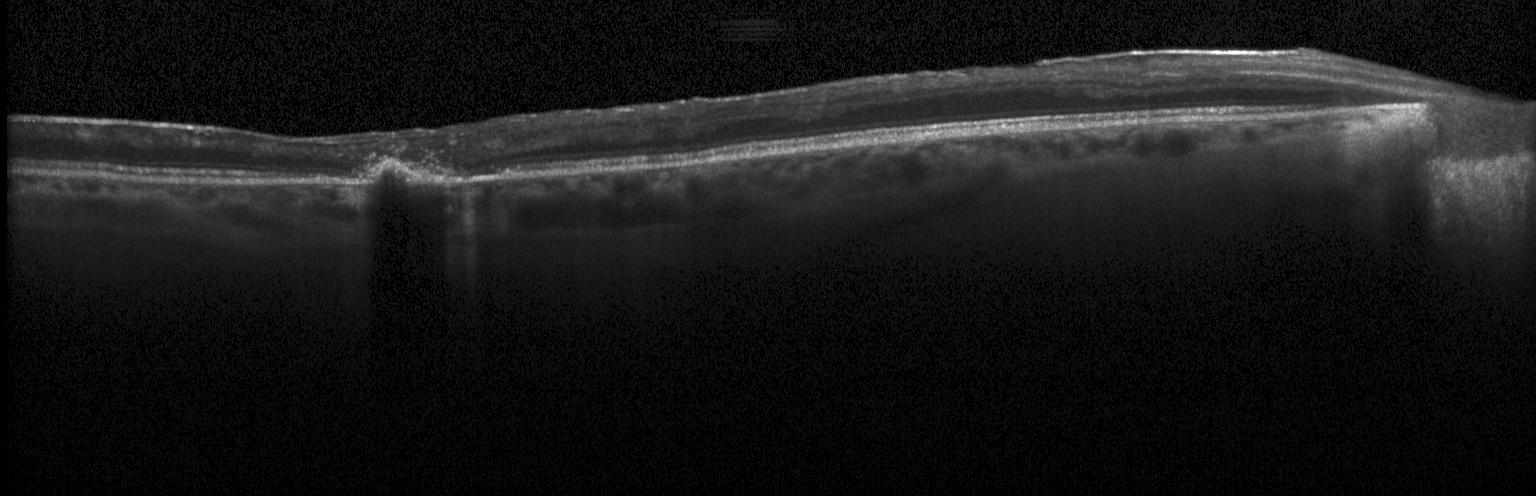 Heidelberg Spectralis OCT system; OCT line scan.
This B-scan demonstrates a choroidal neovascular membrane.